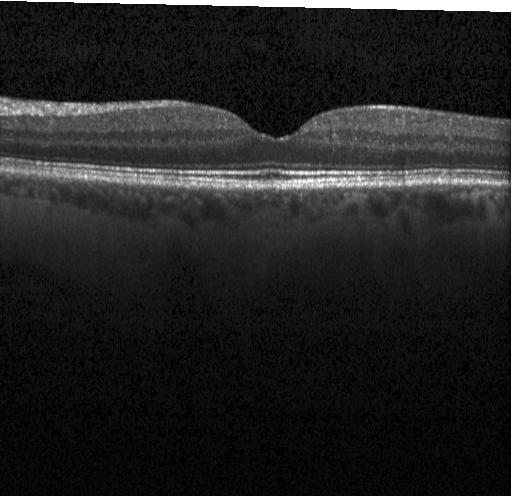
Finding: neither CNV, DME, nor drusen.